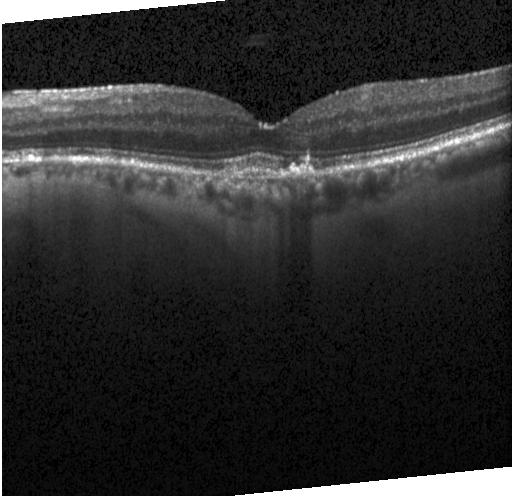
Optical coherence tomography scan, instrument: Heidelberg Spectralis, horizontal scan through the fovea, spectral-domain optical coherence tomography
Finding: a choroidal neovascular membrane.